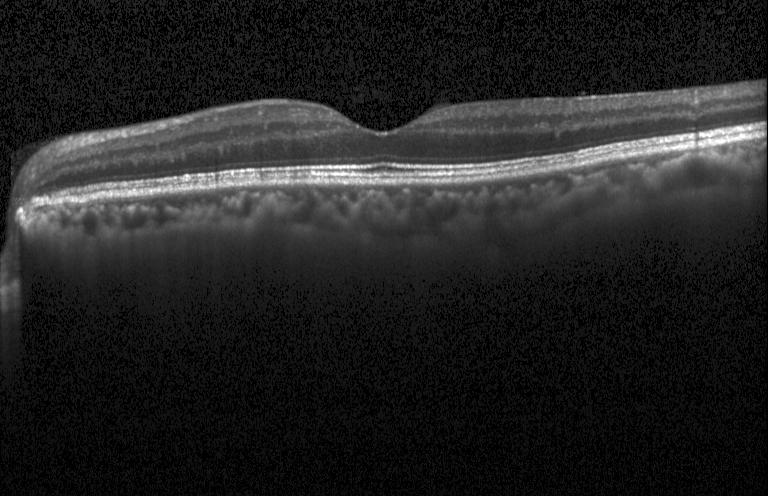
Centered on the fovea; OCT B-scan; SD-OCT.
The scan shows neither CNV, DME, nor drusen.